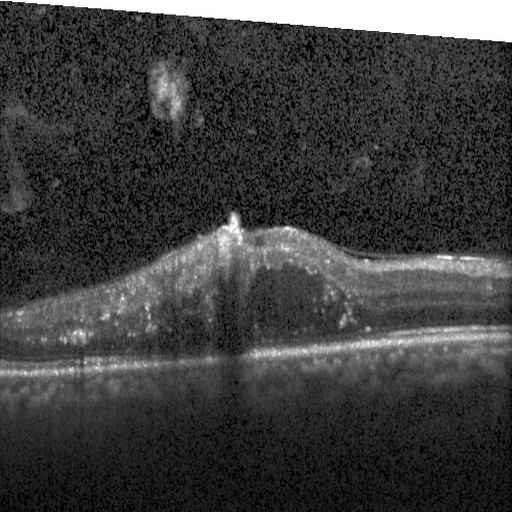
Diabetic macular edema (DME).